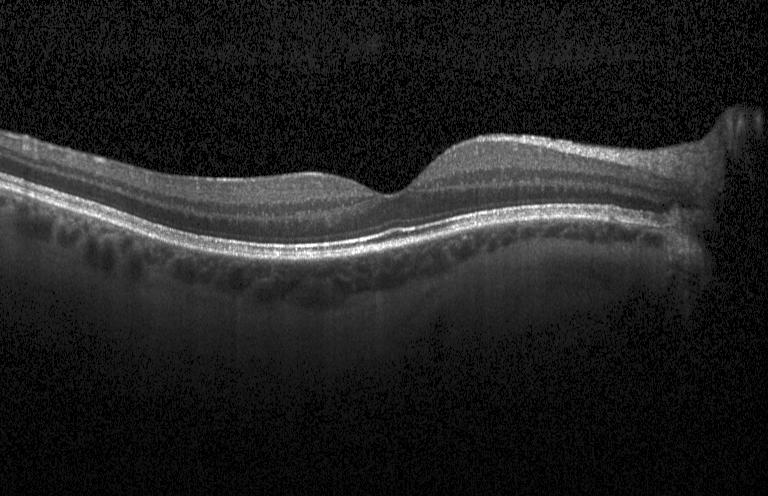
The scan shows no choroidal neovascularization, diabetic macular edema, or drusen.